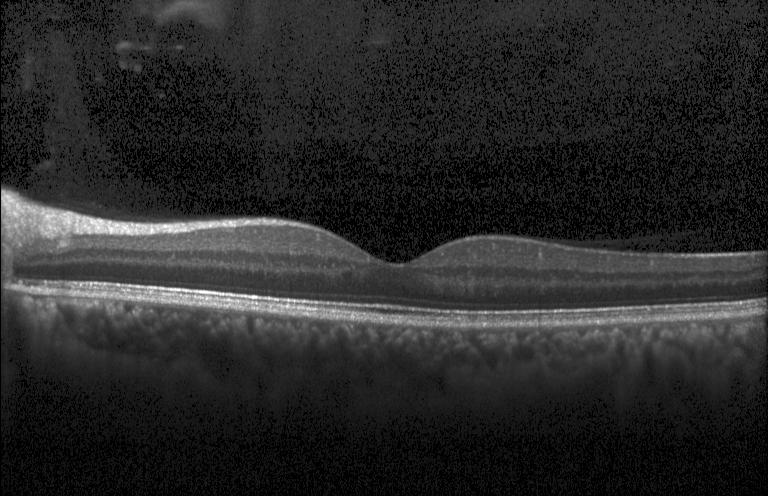

Fovea-centered · optical coherence tomography B-scan · spectral-domain OCT
Diagnosis: no evidence of choroidal neovascularization, diabetic macular edema, or drusen.